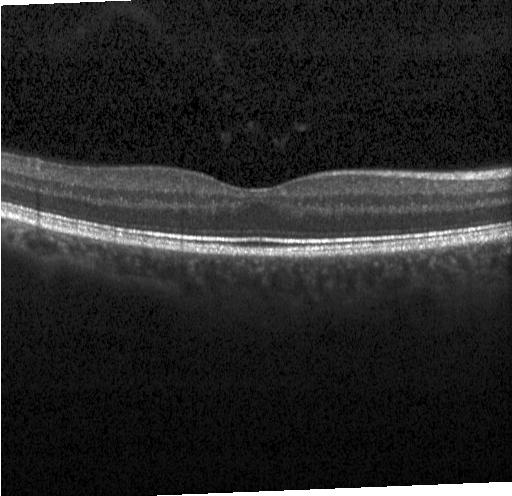
OCT line scan, SD-OCT. The scan shows no choroidal neovascularization, no diabetic macular edema, and no drusen.